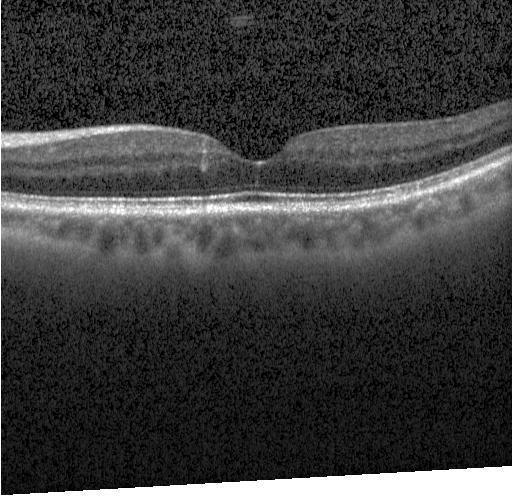
SD-OCT · macular scan · Heidelberg Spectralis OCT system · optical coherence tomography scan
Impression: no choroidal neovascularization, no diabetic macular edema, and no drusen.